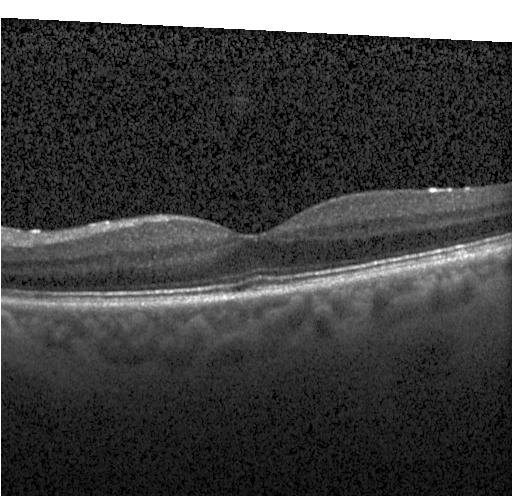

Heidelberg Spectralis, spectral-domain OCT, retinal OCT cross-section. Macular OCT: no evidence of choroidal neovascularization, diabetic macular edema, or drusen.